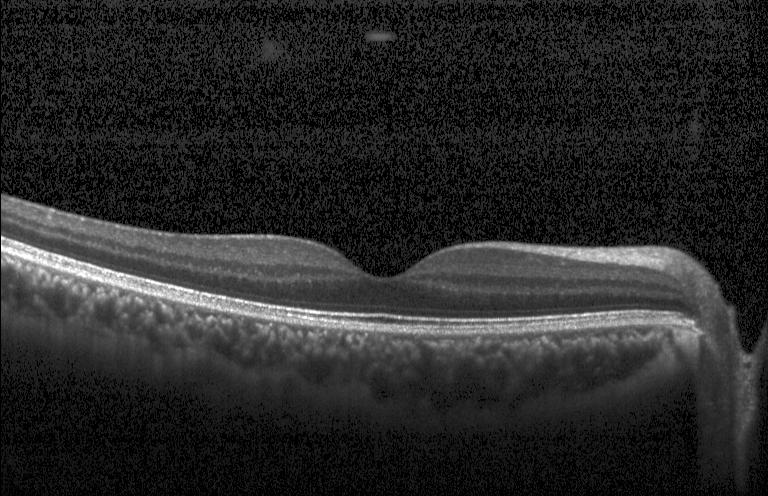

Retinal OCT B-scan; centered on the fovea — Impression: no CNV, DME, or drusen.